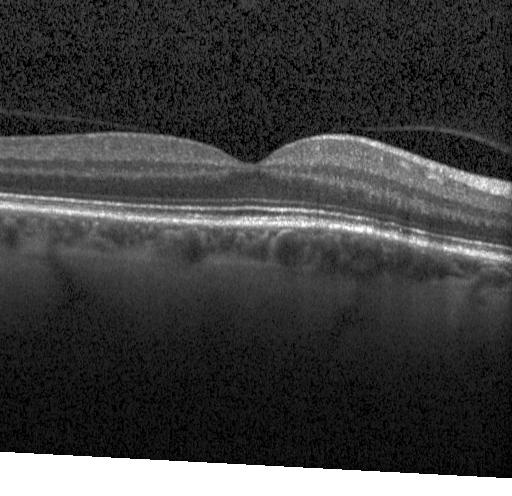
Impression: no choroidal neovascularization, no diabetic macular edema, and no drusen.